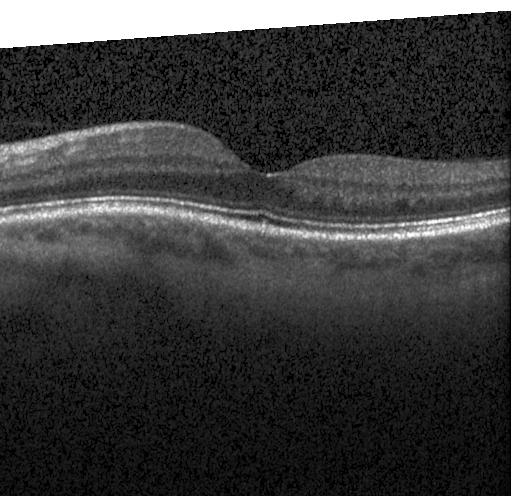

Optical coherence tomography scan · SD-OCT — Diagnosis: neither choroidal neovascularization, diabetic macular edema, nor drusen.